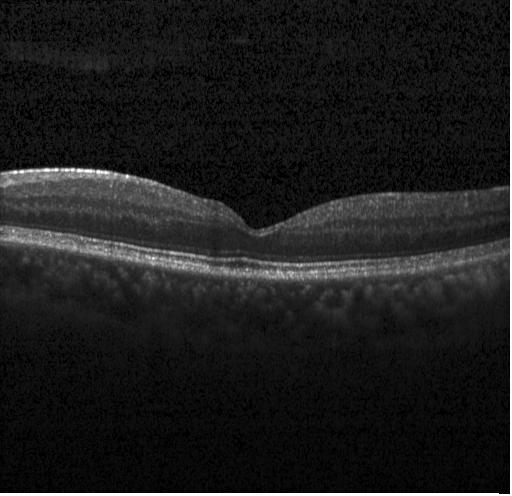

Optical coherence tomography scan. SD-OCT
Finding: no choroidal neovascularization, no diabetic macular edema, and no drusen.